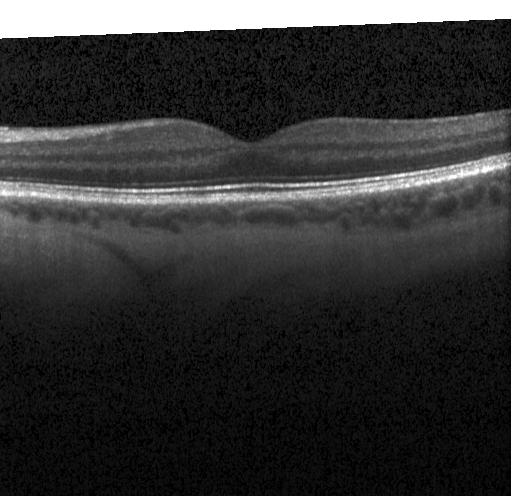

Macular scan. Optical coherence tomography scan. Acquired on a Heidelberg Spectralis. SD-OCT
Impression: no CNV, DME, or drusen.